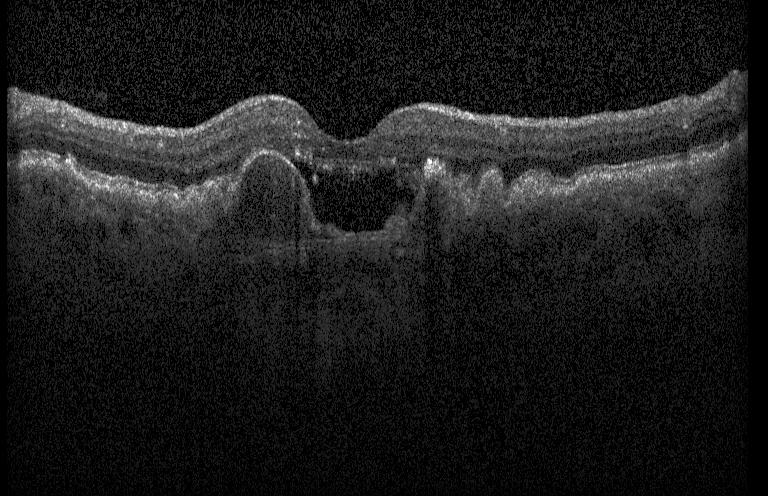

Through the macula · retinal OCT cross-section · SD-OCT.
The scan shows a choroidal neovascular membrane.